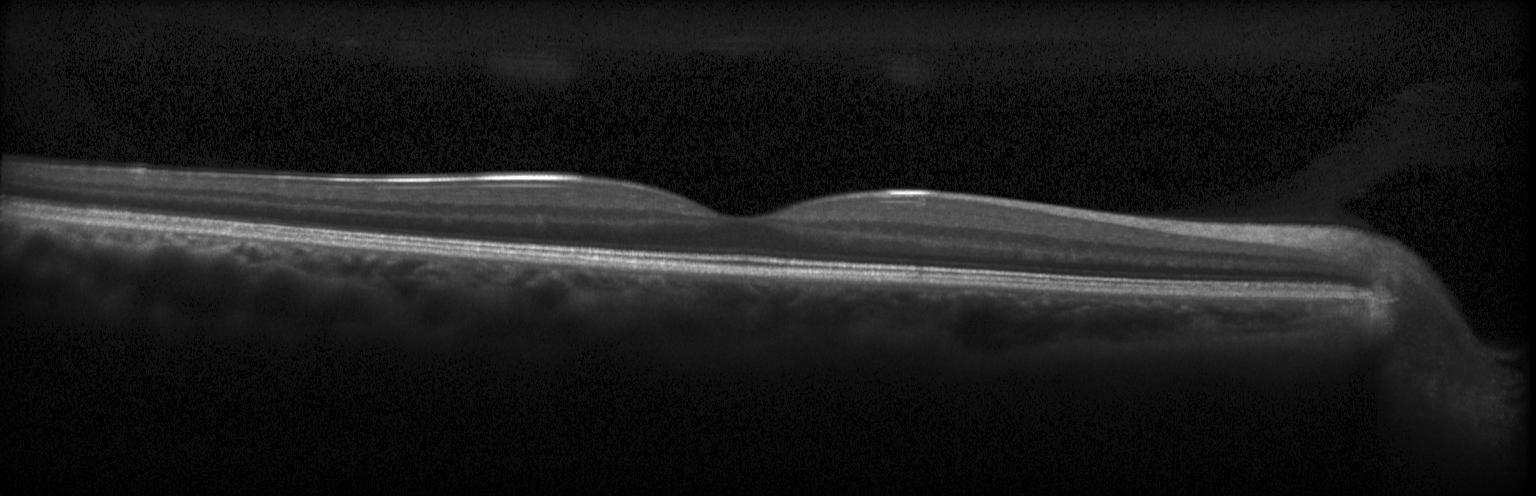 Diagnosis: no evidence of choroidal neovascularization, diabetic macular edema, or drusen.